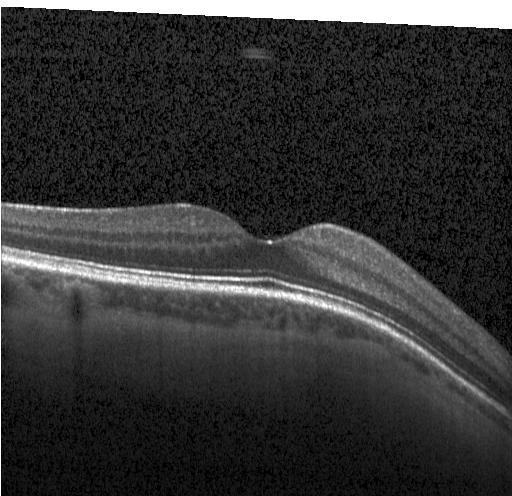 Diagnosis: no choroidal neovascularization, diabetic macular edema, or drusen.